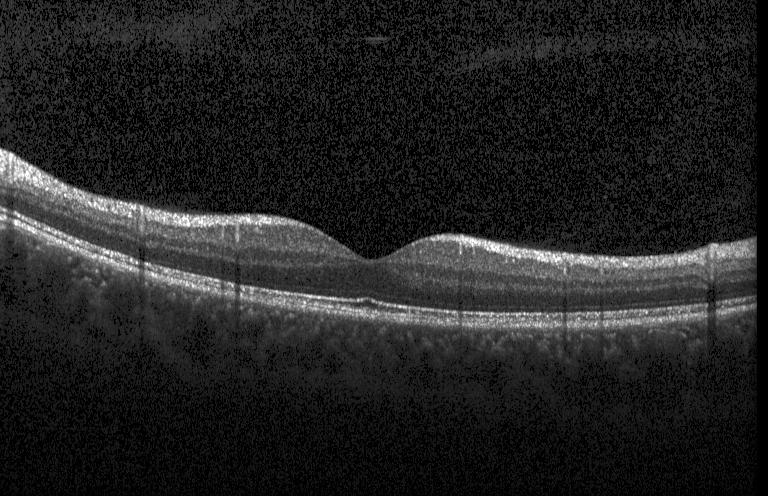
Spectral-domain OCT B-scan: no evidence of choroidal neovascularization, diabetic macular edema, or drusen.